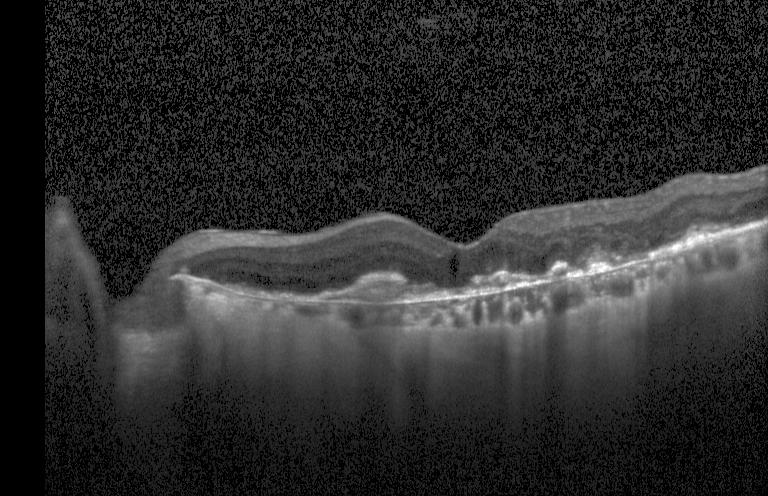 Finding: a choroidal neovascular membrane.